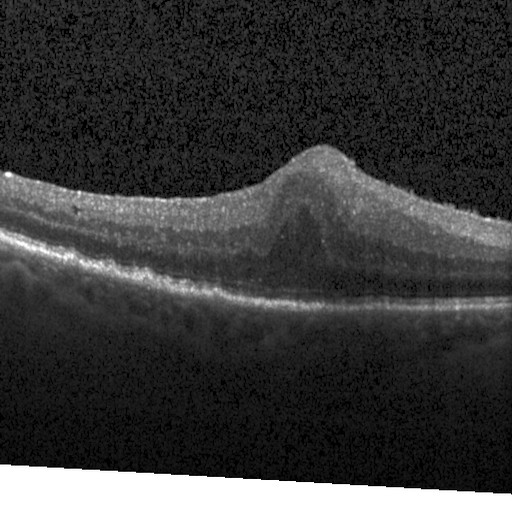
OCT line scan.
Diabetic macular edema (DME).